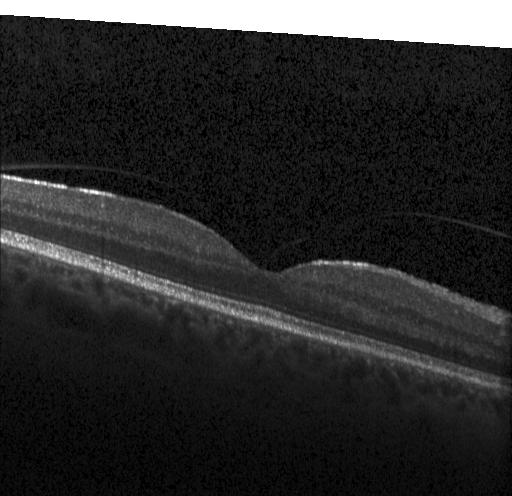
This B-scan demonstrates no CNV, no DME, and no drusen.